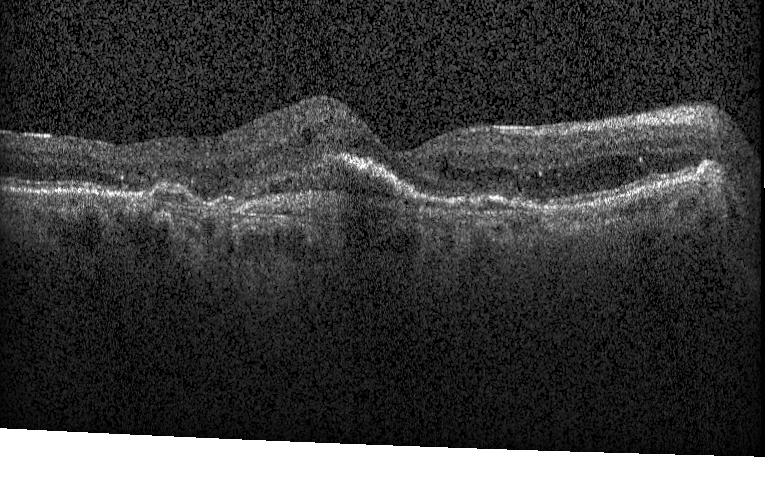 Instrument: Heidelberg Spectralis, retinal OCT cross-section.
Dx: a choroidal neovascular membrane.